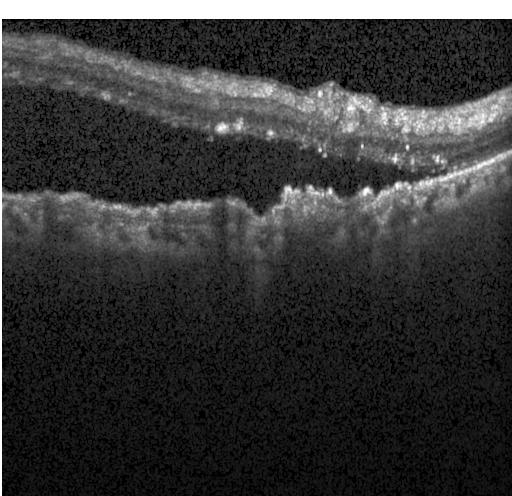
Optical coherence tomography B-scan; Heidelberg Spectralis OCT system. Diagnosis: choroidal neovascularization (CNV).